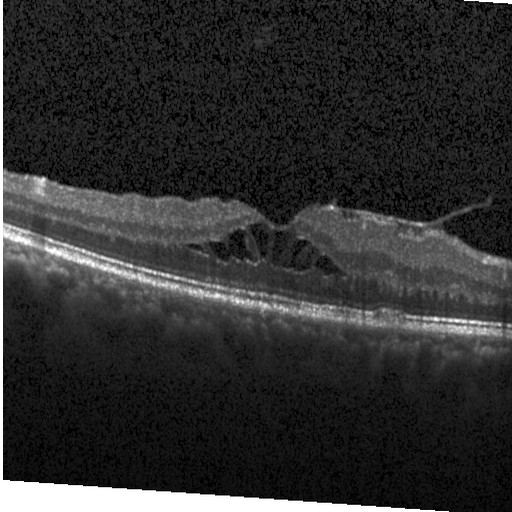
Heidelberg Spectralis · fovea-centered · spectral-domain optical coherence tomography · retinal OCT B-scan — Impression: diabetic macular edema.